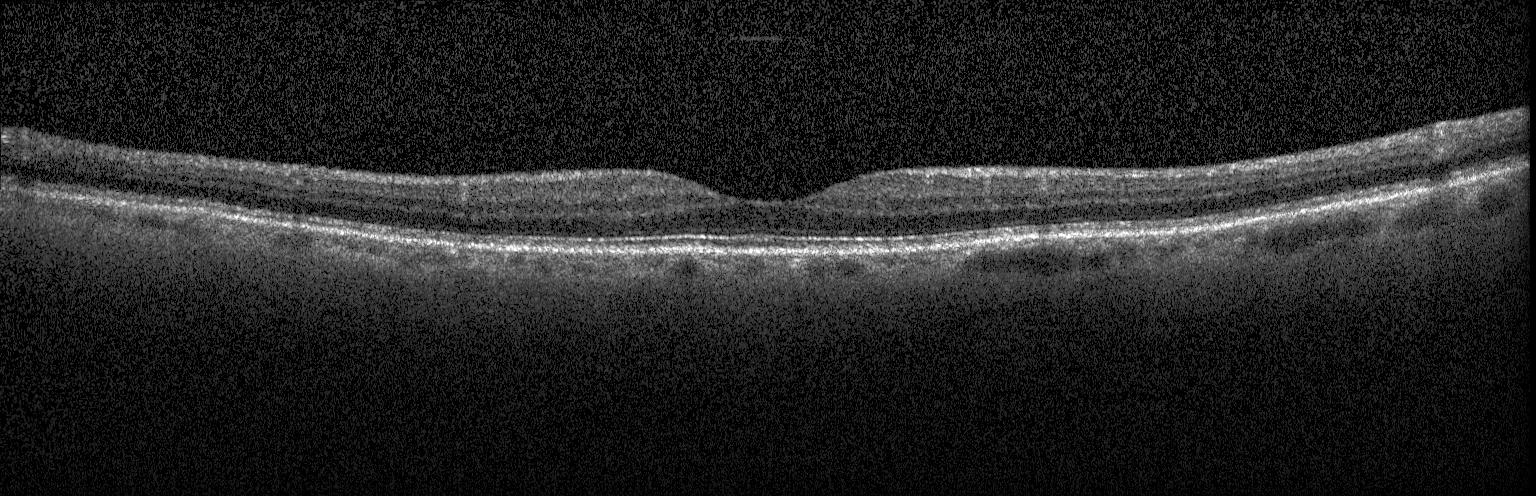
Spectral-domain OCT B-scan: no choroidal neovascularization, diabetic macular edema, or drusen.